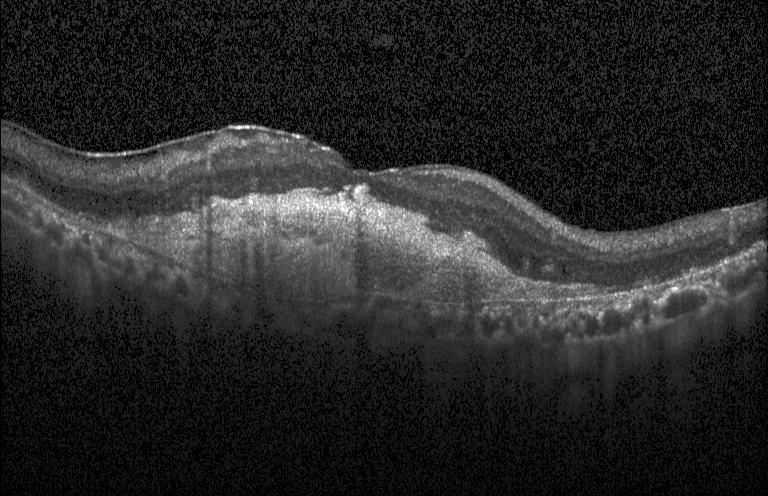
Optical coherence tomography B-scan.
A choroidal neovascular membrane.